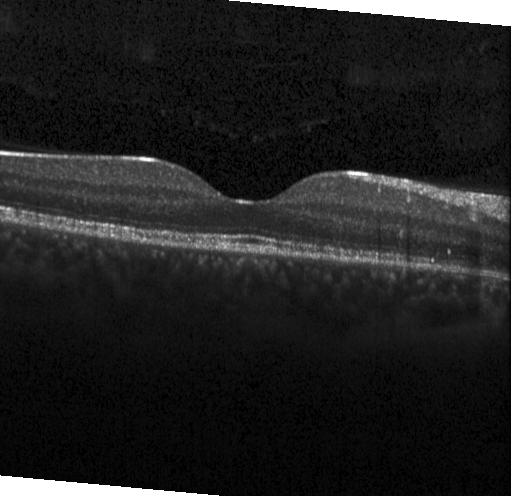
Optical coherence tomography scan, SD-OCT, instrument: Heidelberg Spectralis.
OCT finding: no evidence of CNV, DME, or drusen.